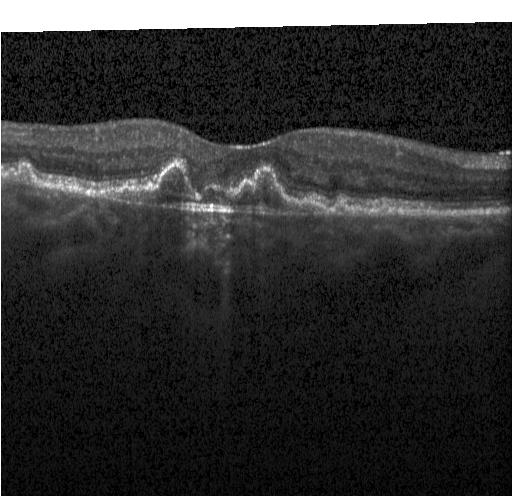
Macular OCT demonstrating choroidal neovascularization.